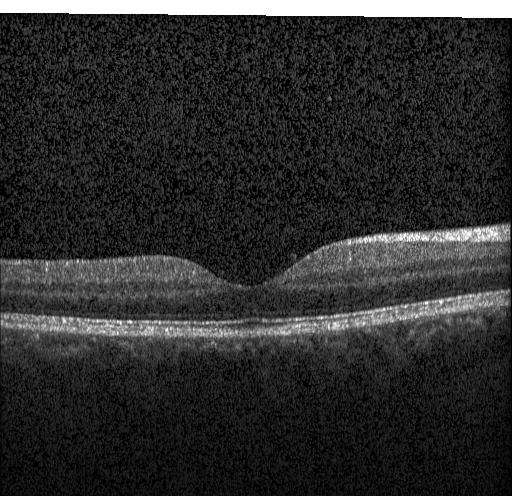
Spectral-domain OCT B-scan: no CNV, no DME, and no drusen.